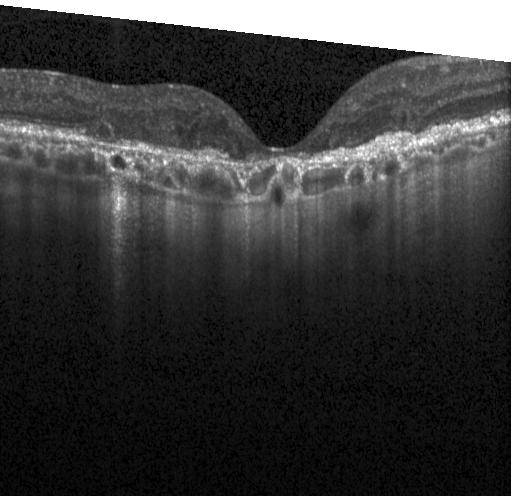 Heidelberg Spectralis · optical coherence tomography B-scan
OCT finding: a choroidal neovascular membrane.